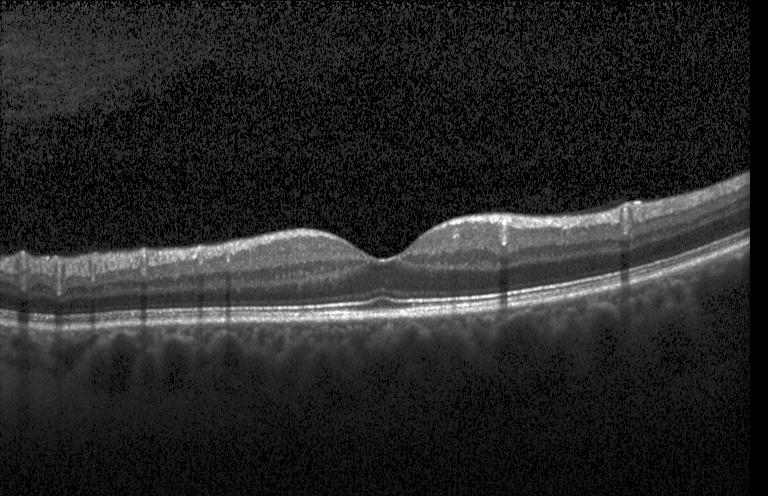 Retinal OCT cross-section. Diagnosis: no choroidal neovascularization, diabetic macular edema, or drusen.